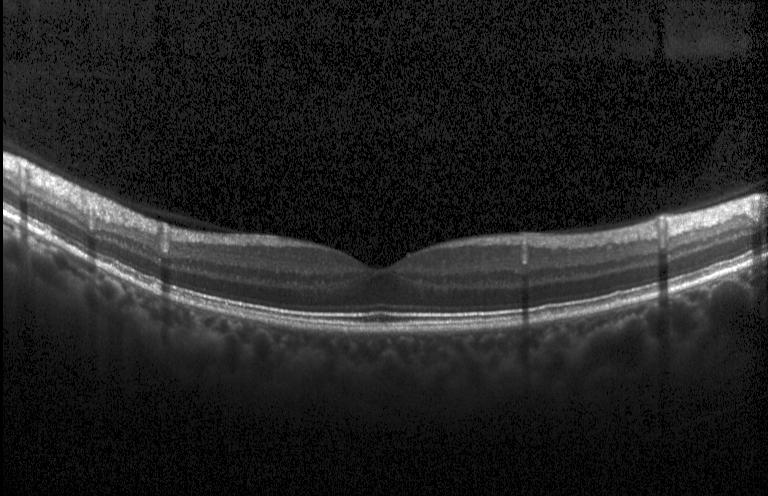
Spectral-domain OCT, OCT line scan, acquired on a Heidelberg Spectralis.
Assessment: no CNV, no DME, and no drusen.